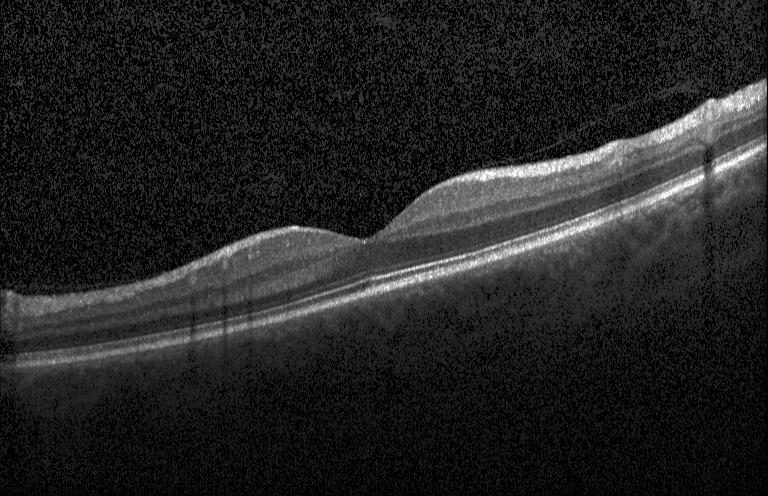 OCT line scan, spectral-domain optical coherence tomography, horizontal scan through the fovea. This B-scan demonstrates no choroidal neovascularization, diabetic macular edema, or drusen.